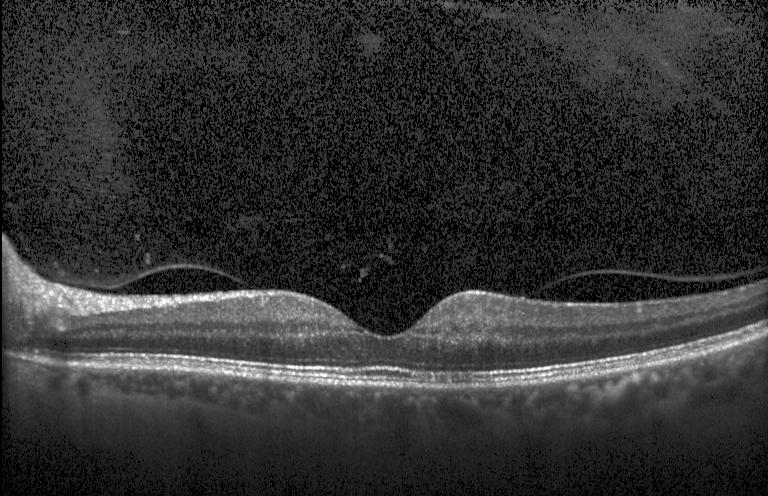

Optical coherence tomography scan, acquired on a Heidelberg Spectralis, spectral-domain optical coherence tomography.
Dx: no evidence of choroidal neovascularization, diabetic macular edema, or drusen.